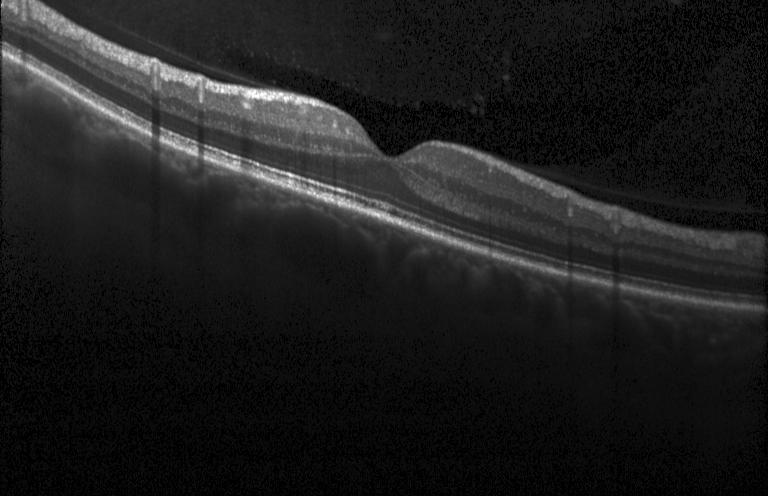
Heidelberg Spectralis. OCT line scan. Spectral-domain optical coherence tomography. Horizontal scan through the fovea.
Finding: no evidence of CNV, DME, or drusen.